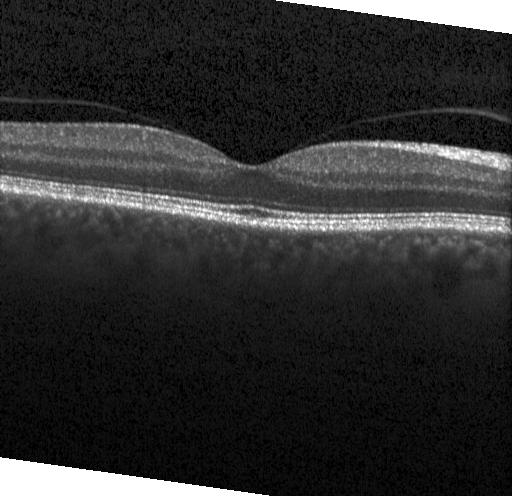
Acquired on a Heidelberg Spectralis; macular scan; optical coherence tomography scan
Diagnosis: no choroidal neovascularization, no diabetic macular edema, and no drusen.